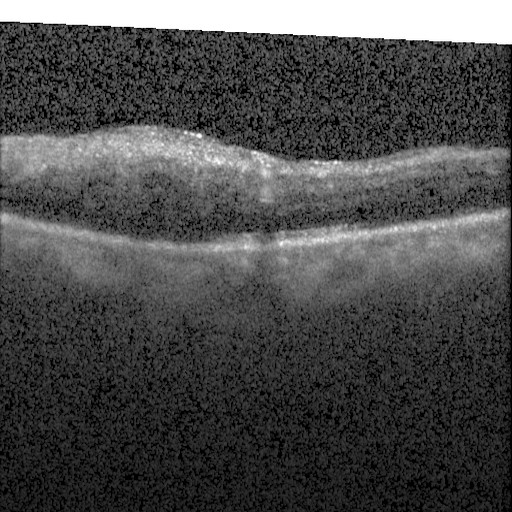
OCT finding: diabetic macular edema.